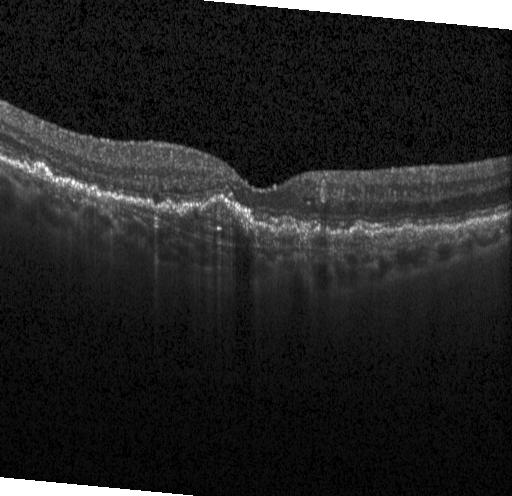

Fovea-centered; optical coherence tomography B-scan.
Finding: choroidal neovascularization (CNV).